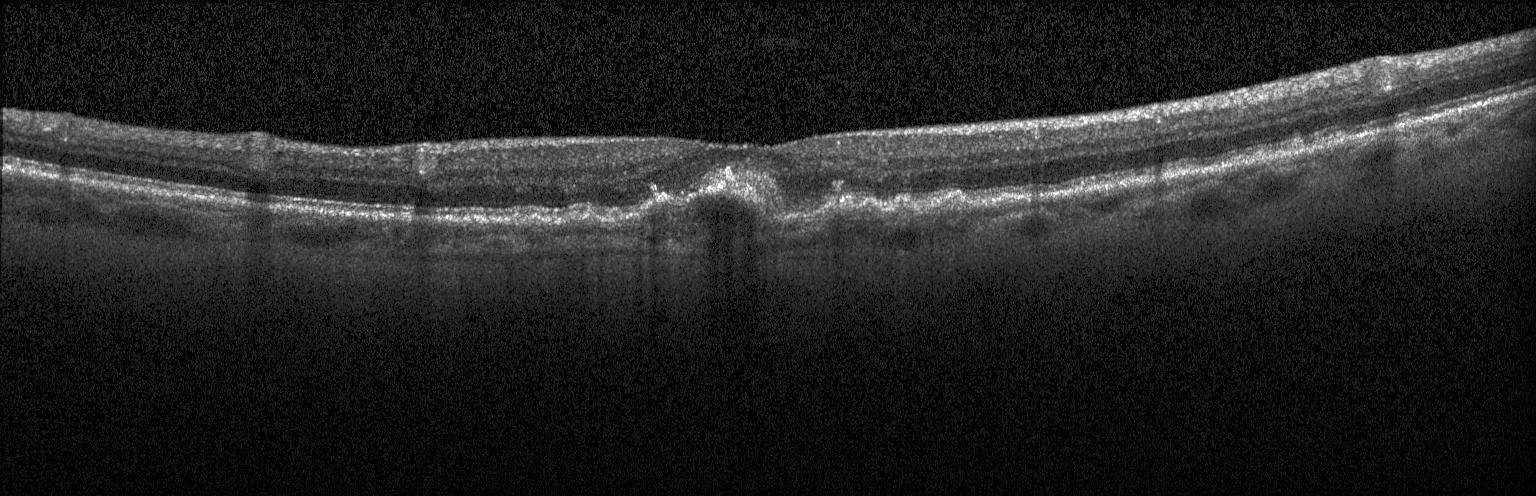

SD-OCT, through the macula, retinal OCT cross-section
A choroidal neovascular membrane.